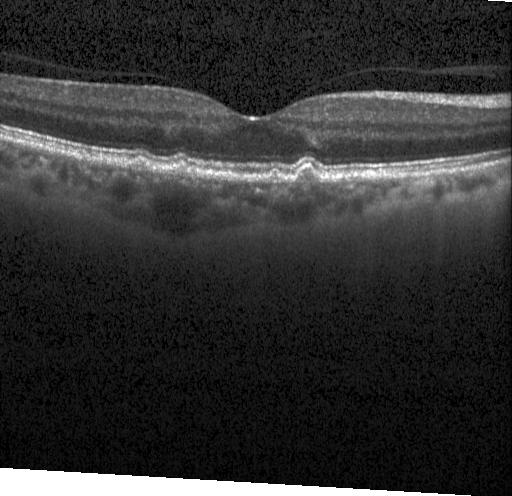
OCT line scan · fovea-centered
Diagnosis: multiple drusen.